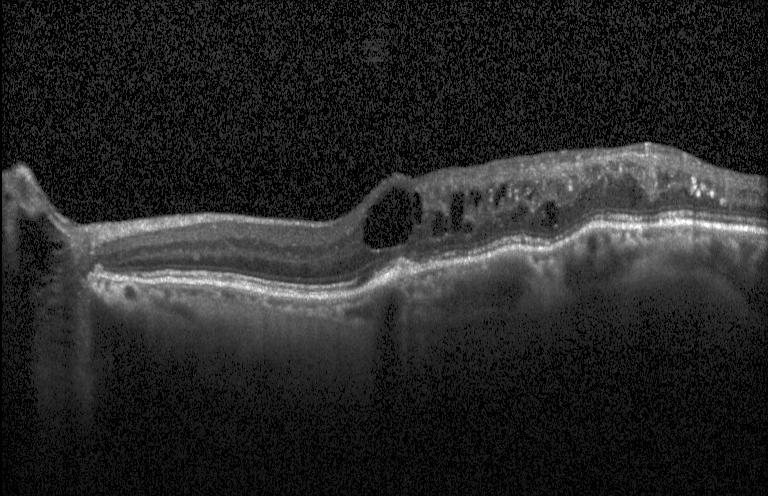
Acquired on a Heidelberg Spectralis, macular scan, spectral-domain optical coherence tomography, OCT line scan — Impression: DME.